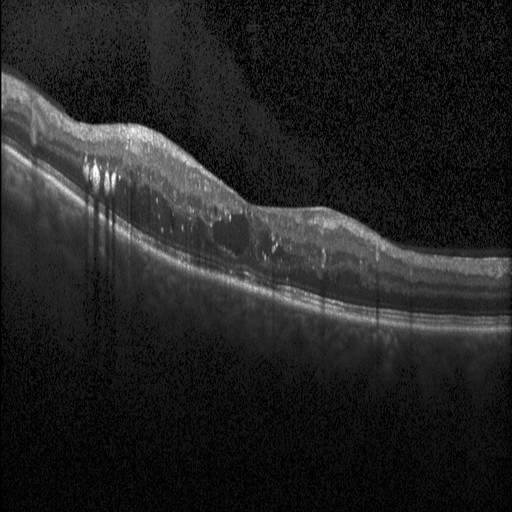

Diagnosis: DME.